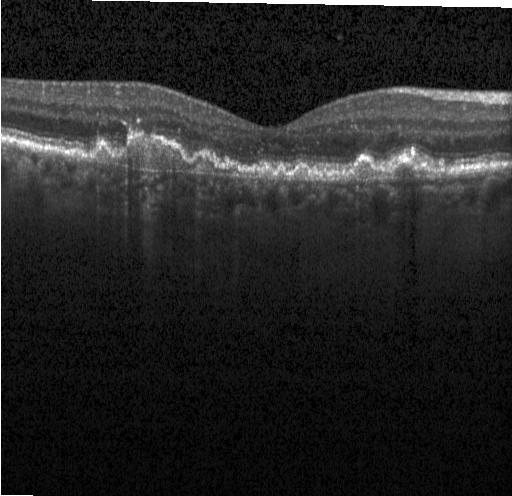

SD-OCT · instrument: Heidelberg Spectralis · OCT B-scan · through the macula — Impression: choroidal neovascularization.